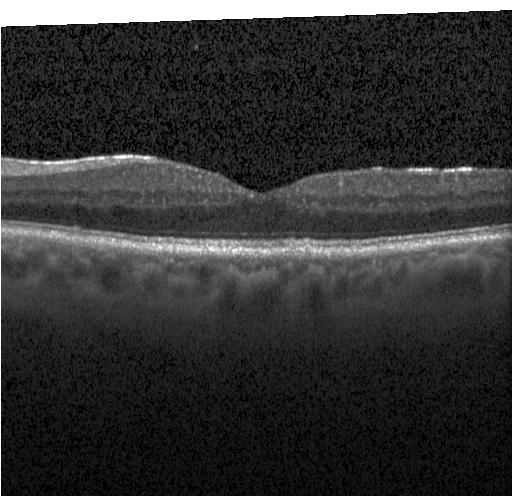 OCT line scan — Impression: neither CNV, DME, nor drusen.